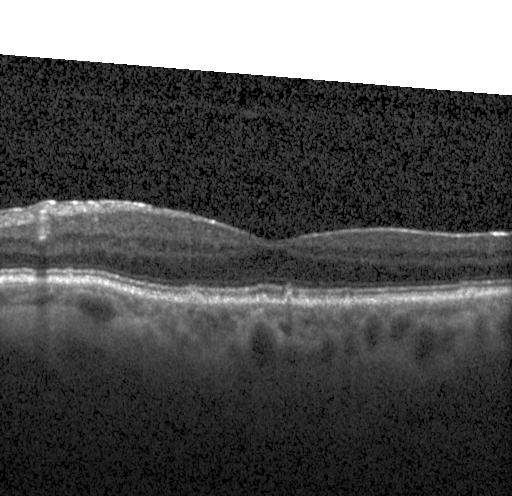
OCT finding: sub-RPE drusenoid deposits.